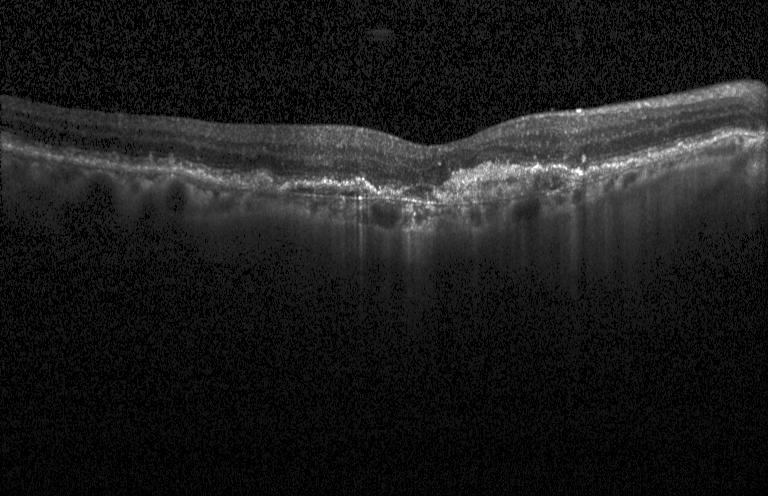

OCT line scan. Diagnosis: a choroidal neovascular membrane.